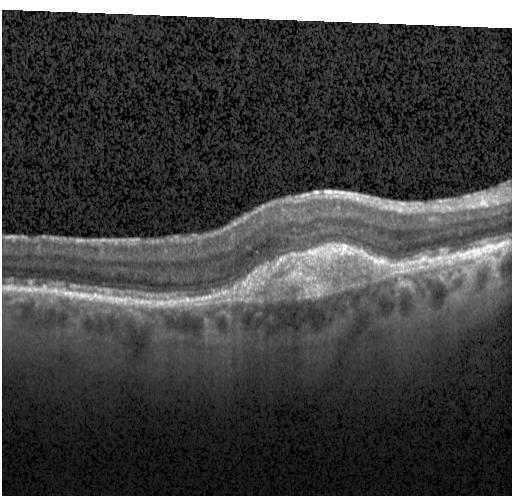

OCT scan showing choroidal neovascularization.